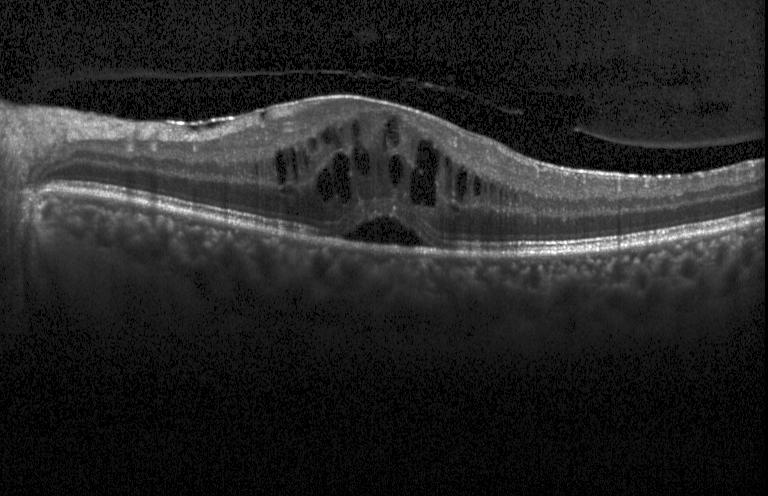
Retinal OCT cross-section; centered on the fovea. Diagnosis: diabetic macular edema.